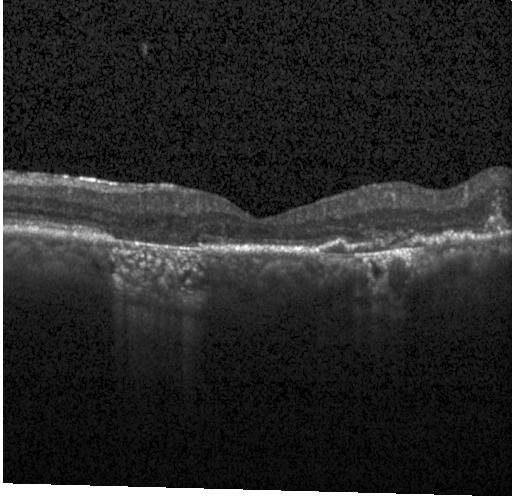 OCT finding: CNV.